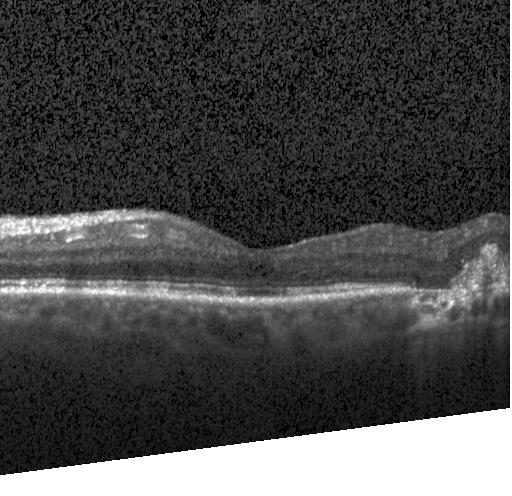
Instrument: Heidelberg Spectralis, optical coherence tomography scan, horizontal scan through the fovea.
A choroidal neovascular membrane.